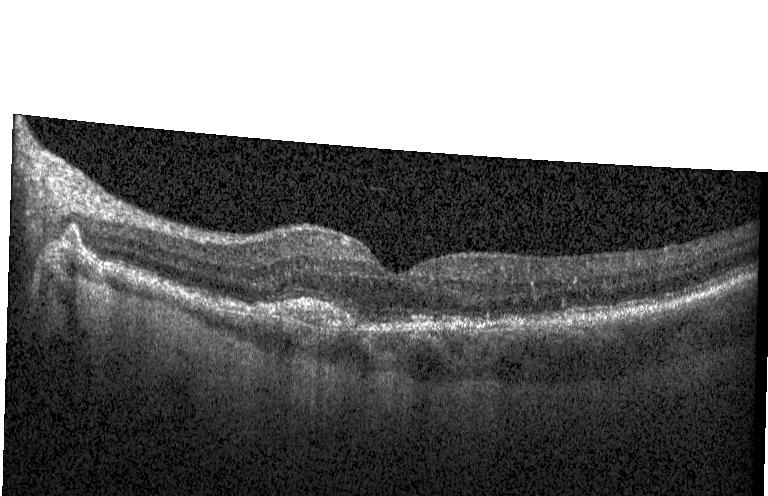 CNV.